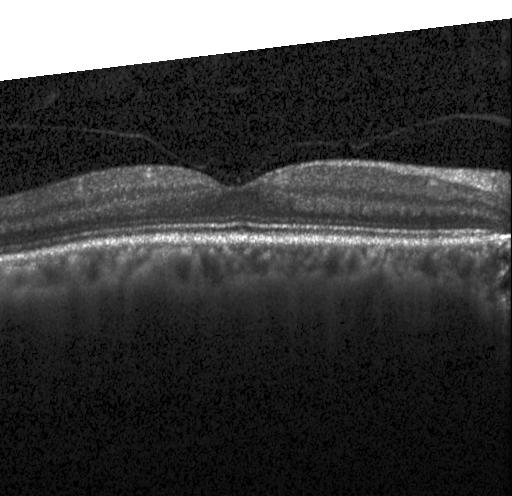 OCT B-scan showing no evidence of choroidal neovascularization, diabetic macular edema, or drusen.